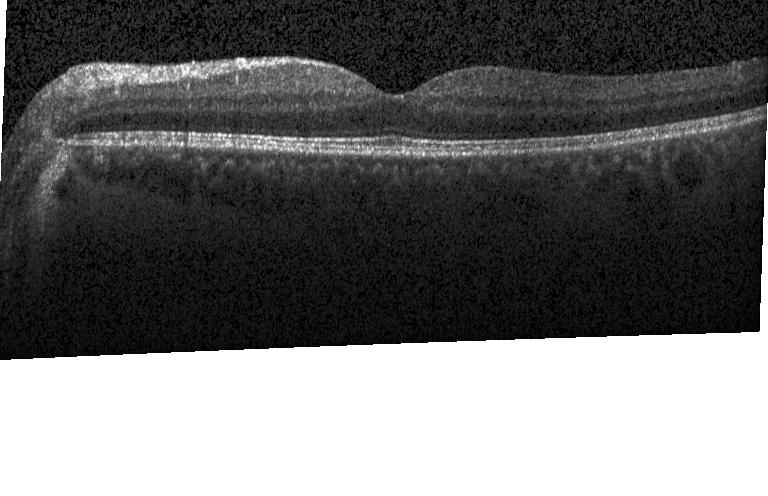 Retinal OCT B-scan · spectral-domain OCT · horizontal scan through the fovea · instrument: Heidelberg Spectralis — Finding: neither CNV, DME, nor drusen.